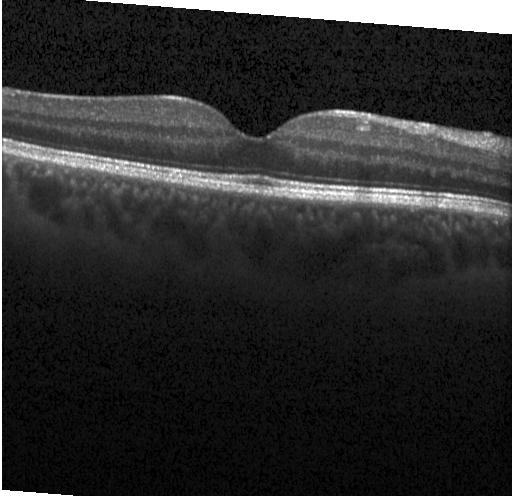 No evidence of CNV, DME, or drusen.